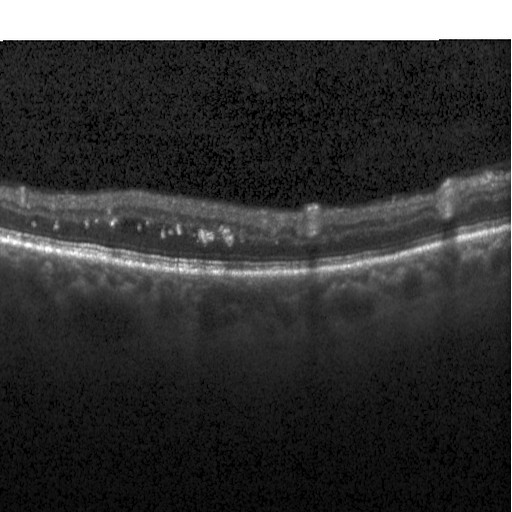
OCT finding: diabetic macular edema (DME).